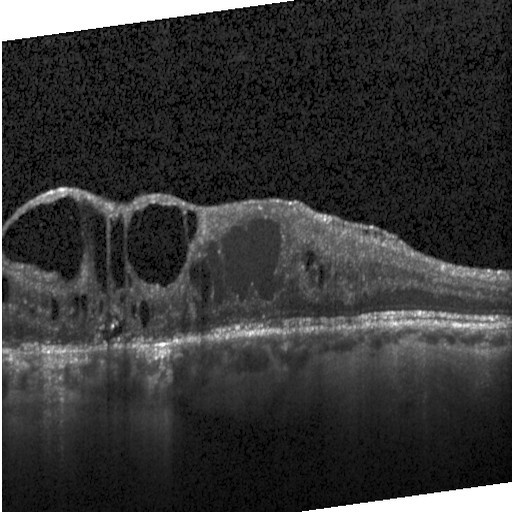
Acquired on a Heidelberg Spectralis · spectral-domain optical coherence tomography · optical coherence tomography B-scan — Impression: DME.